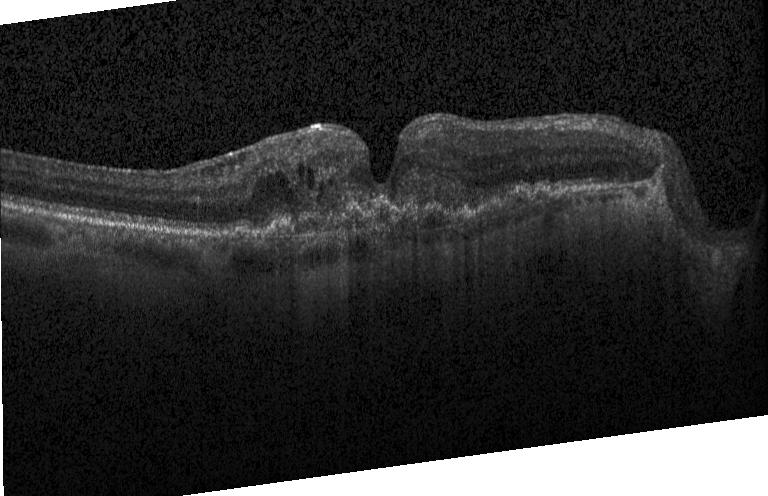

Impression: choroidal neovascularization.